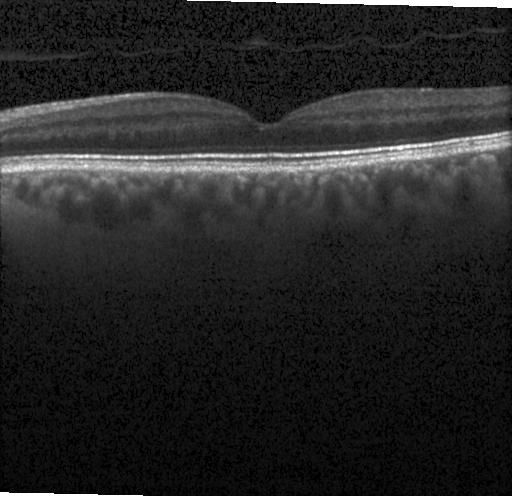

Macular OCT: no choroidal neovascularization, no diabetic macular edema, and no drusen.